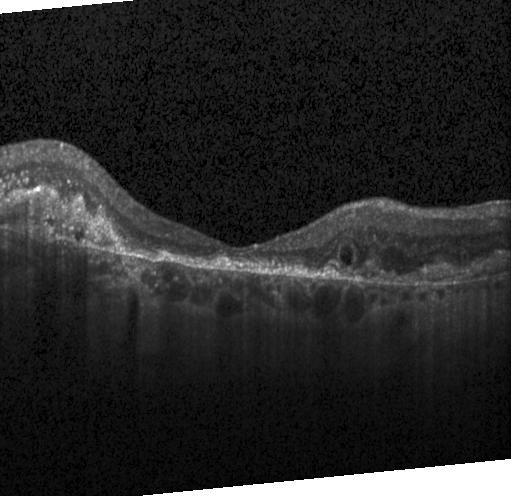 Spectral-domain OCT B-scan: a choroidal neovascular membrane.